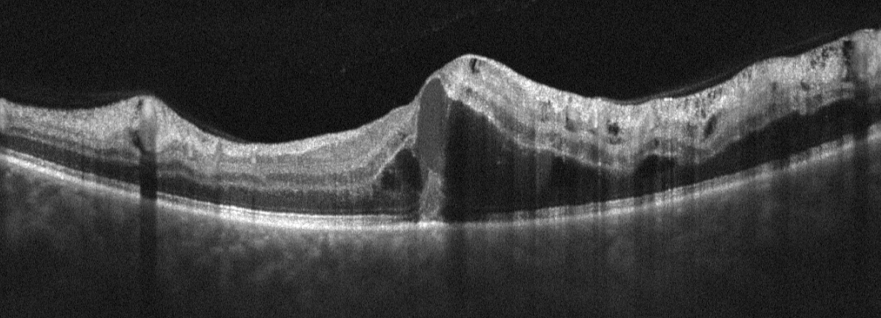

Impression: RVO.